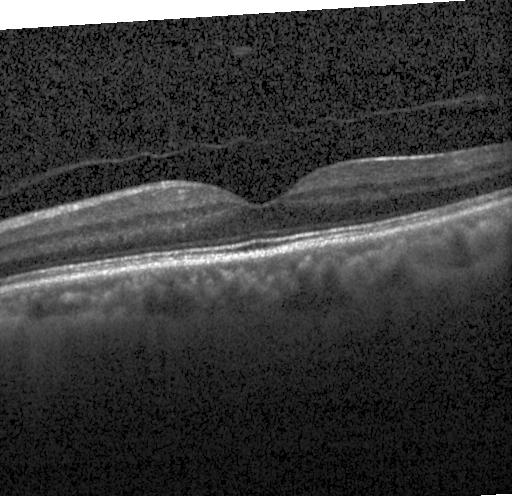

OCT B-scan.
Neither CNV, DME, nor drusen.